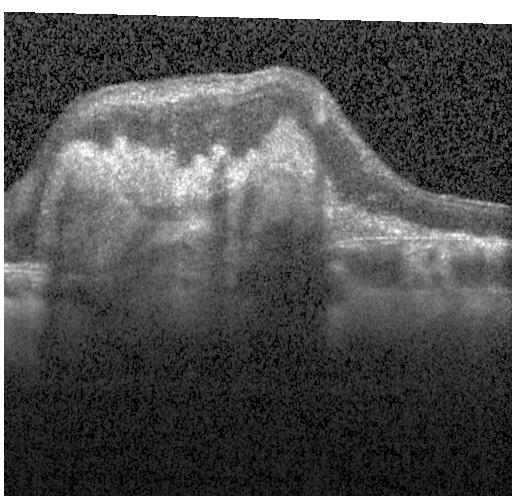
Heidelberg Spectralis · OCT B-scan · macular scan · spectral-domain optical coherence tomography.
Finding: a choroidal neovascular membrane.